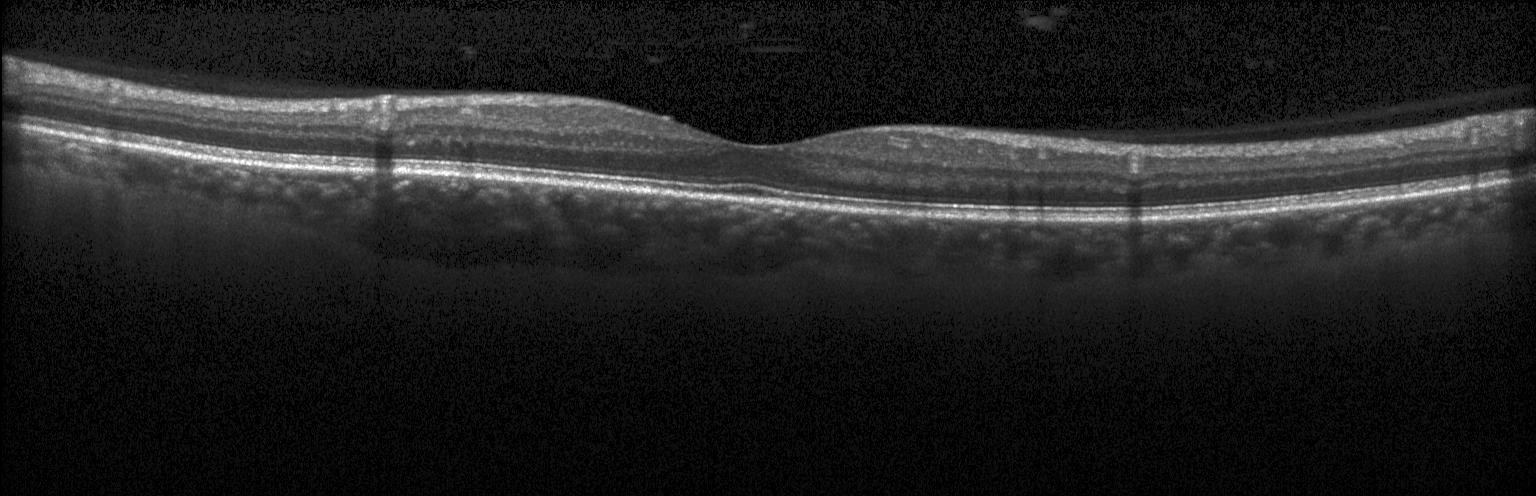

Instrument: Heidelberg Spectralis; retinal OCT cross-section; centered on the fovea
Impression: no evidence of choroidal neovascularization, diabetic macular edema, or drusen.